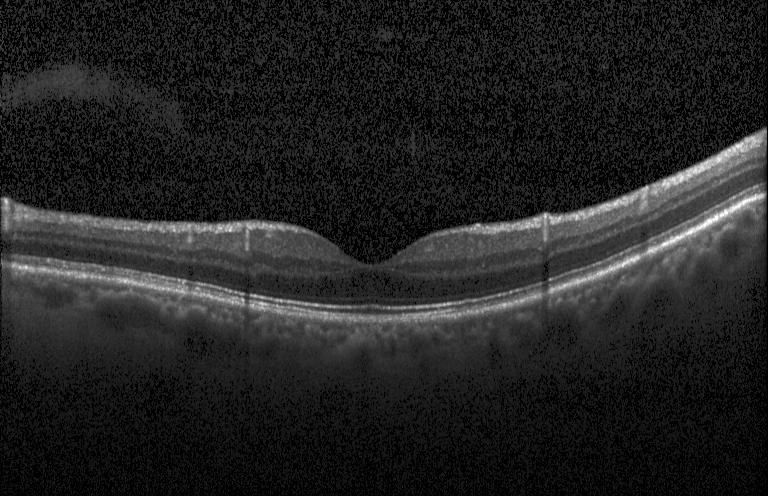

Retinal OCT B-scan · Heidelberg Spectralis · through the macula
Impression: no evidence of choroidal neovascularization, diabetic macular edema, or drusen.